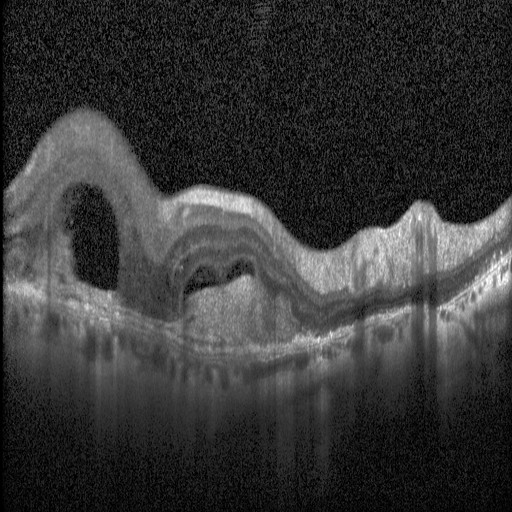
Macular OCT: diabetic macular edema.